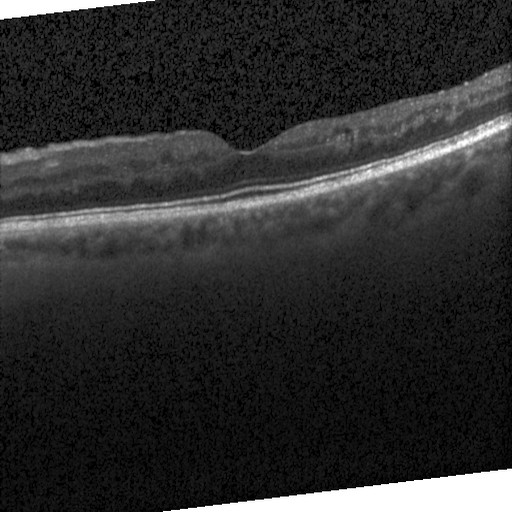 Macular scan; optical coherence tomography scan
Impression: diabetic macular edema.